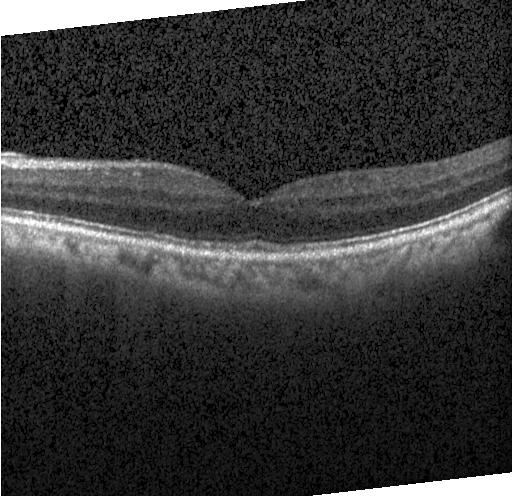 Instrument: Heidelberg Spectralis; optical coherence tomography scan.
OCT finding: no evidence of choroidal neovascularization, diabetic macular edema, or drusen.